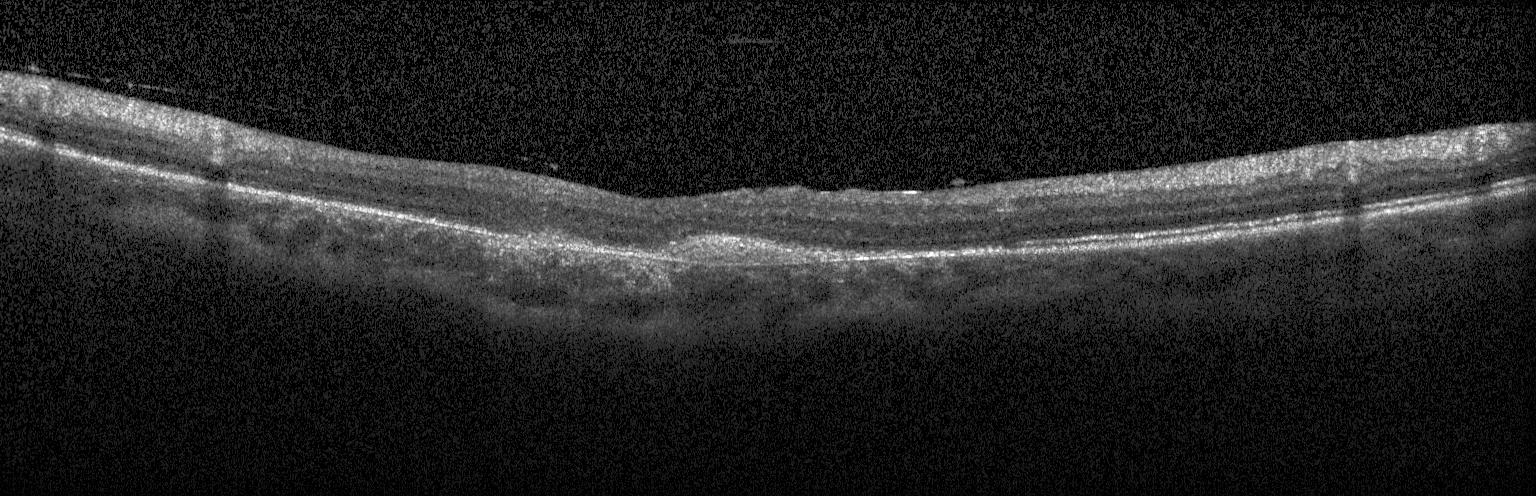
OCT B-scan. Heidelberg Spectralis.
Impression: a choroidal neovascular membrane.